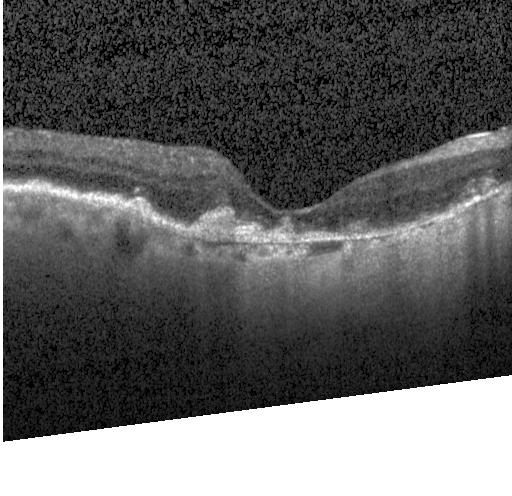

OCT B-scan
This B-scan demonstrates choroidal neovascularization.